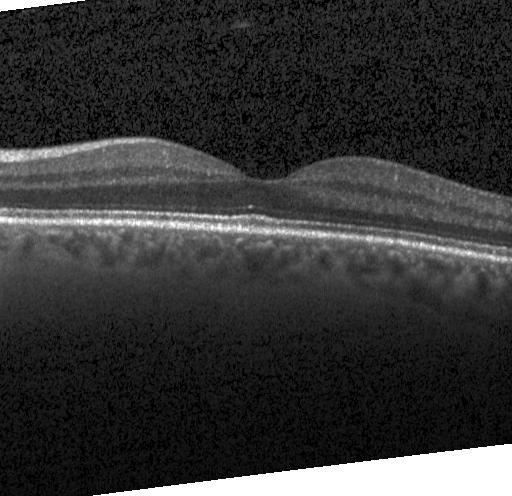
Dx: neither choroidal neovascularization, diabetic macular edema, nor drusen.